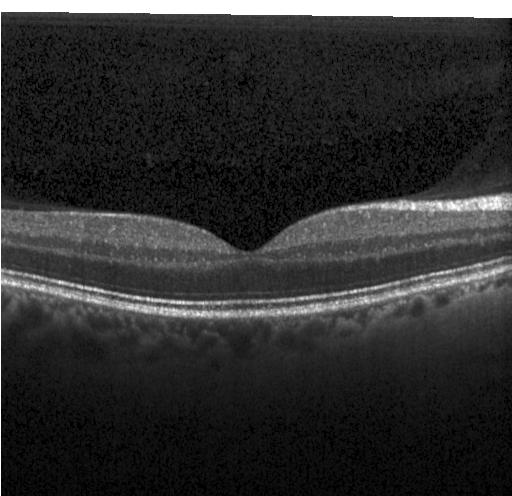 Diagnosis: no CNV, no DME, and no drusen.